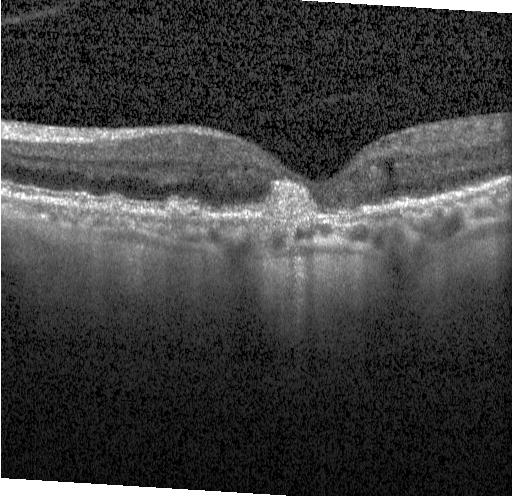 Retinal OCT B-scan. Spectral-domain OCT. Diagnosis: a choroidal neovascular membrane.